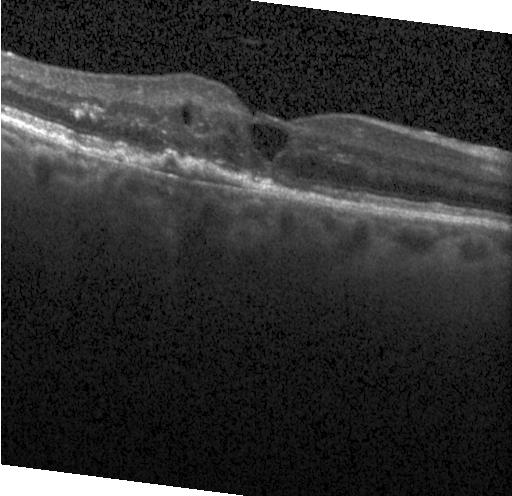

Spectral-domain optical coherence tomography. Macular scan. Retinal OCT B-scan
Finding: a choroidal neovascular membrane.